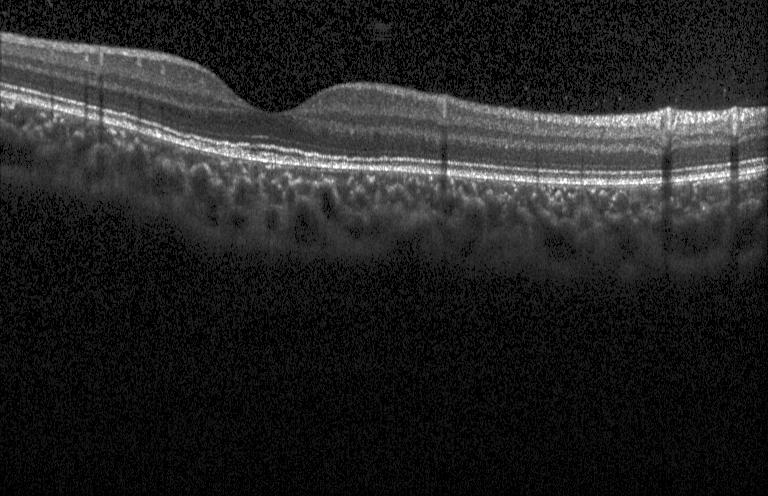

Dx: no evidence of choroidal neovascularization, diabetic macular edema, or drusen.